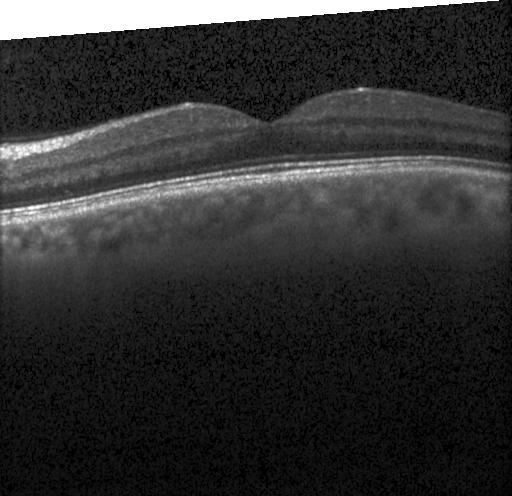 Optical coherence tomography B-scan, SD-OCT. Dx: no CNV, no DME, and no drusen.